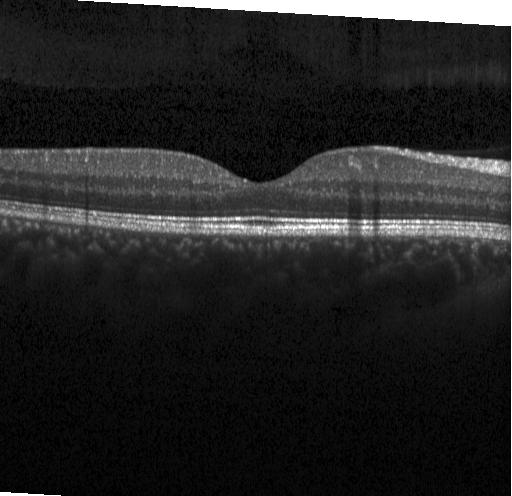

Heidelberg Spectralis, SD-OCT, optical coherence tomography scan. Impression: no evidence of choroidal neovascularization, diabetic macular edema, or drusen.